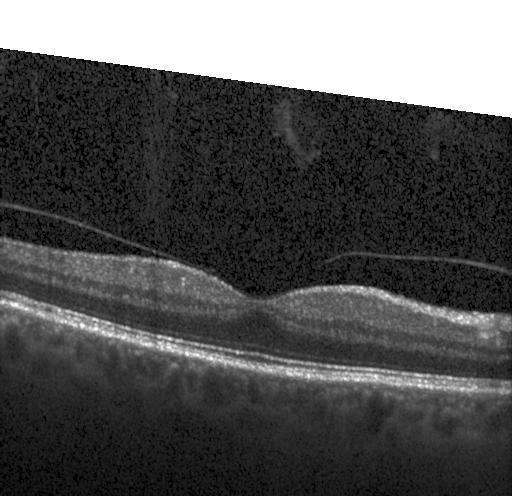 Optical coherence tomography scan
No CNV, no DME, and no drusen.